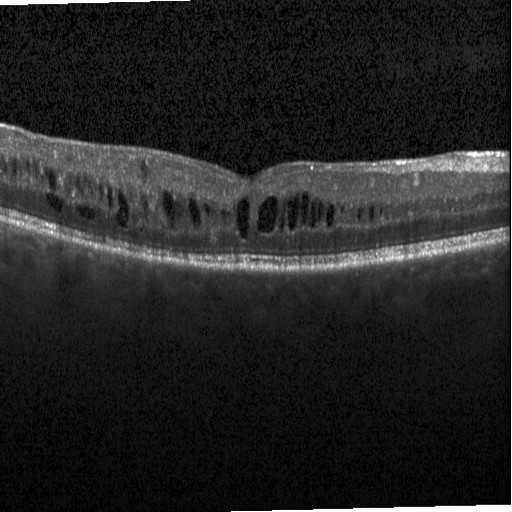
Through the macula · retinal OCT B-scan · Heidelberg Spectralis
Diabetic macular edema.